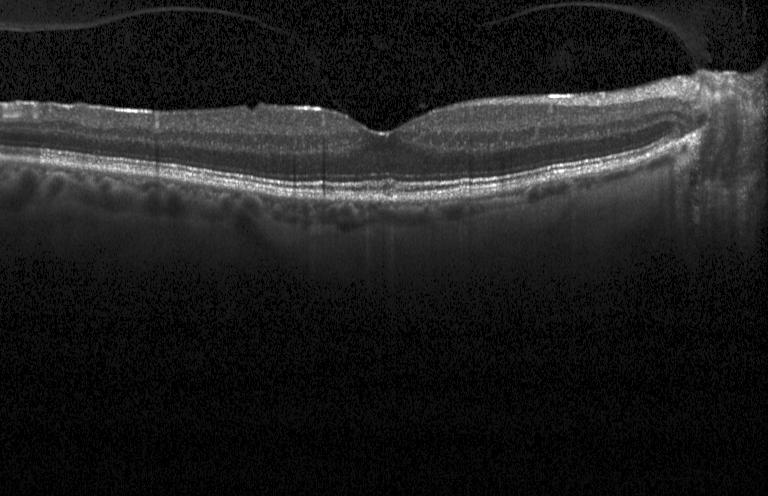
Heidelberg Spectralis, spectral-domain optical coherence tomography, OCT line scan, horizontal scan through the fovea — Neither choroidal neovascularization, diabetic macular edema, nor drusen.